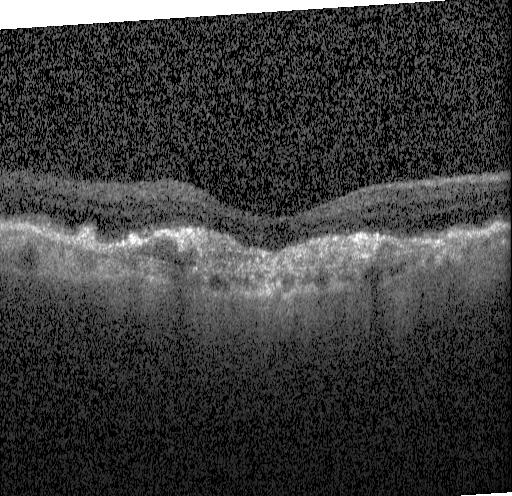 OCT line scan. Heidelberg Spectralis. Spectral-domain OCT. Horizontal scan through the fovea — Diagnosis: CNV.